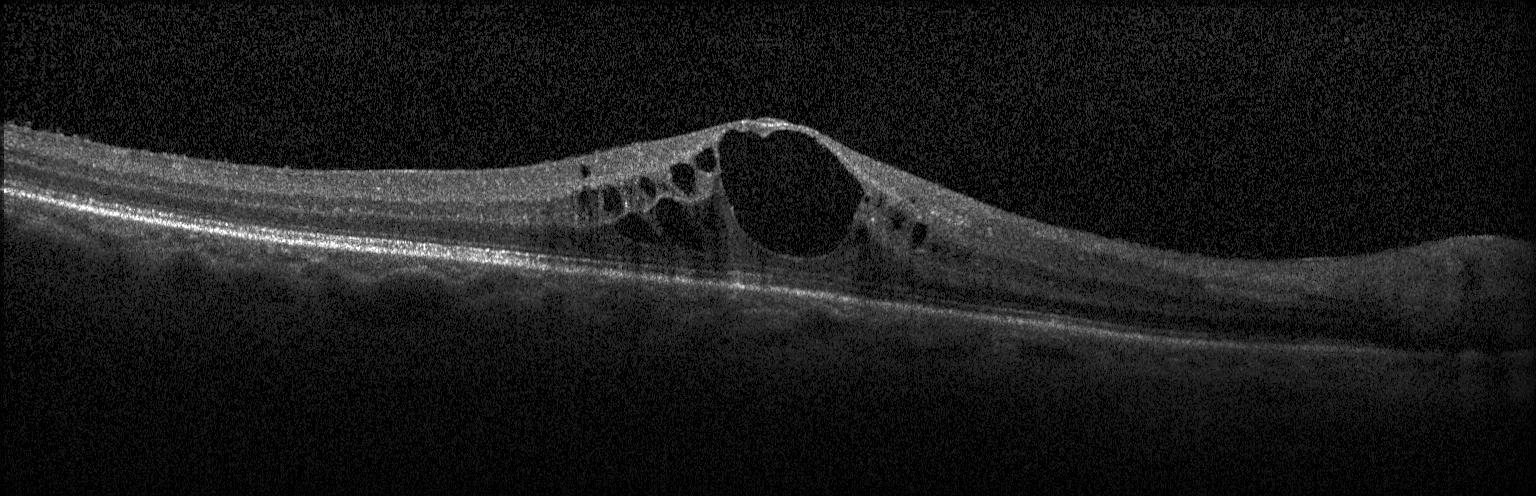
Optical coherence tomography scan — This B-scan demonstrates DME.